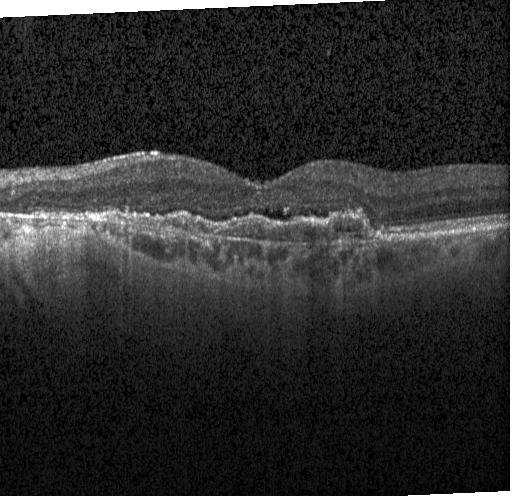

Retinal OCT cross-section · spectral-domain OCT · instrument: Heidelberg Spectralis · macular scan — Impression: choroidal neovascularization.